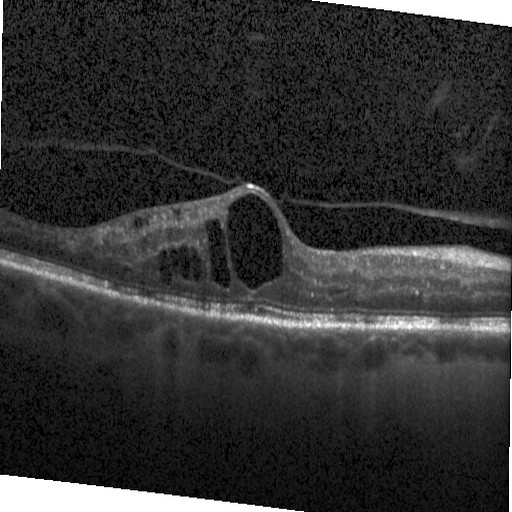
Diagnosis: DME.